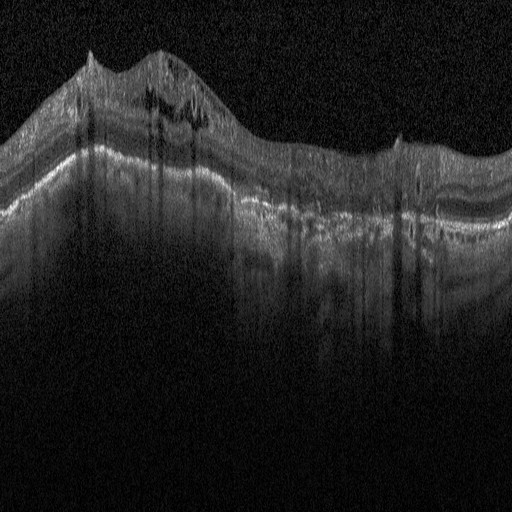

Centered on the fovea · spectral-domain OCT · optical coherence tomography B-scan. Dx: DME.